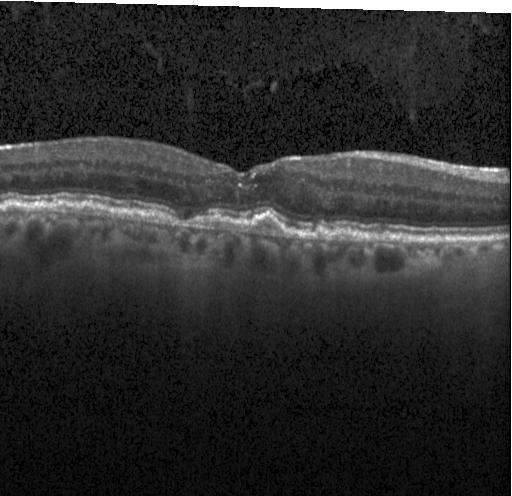

Macular scan, spectral-domain OCT, OCT B-scan.
Impression: choroidal neovascularization (CNV).